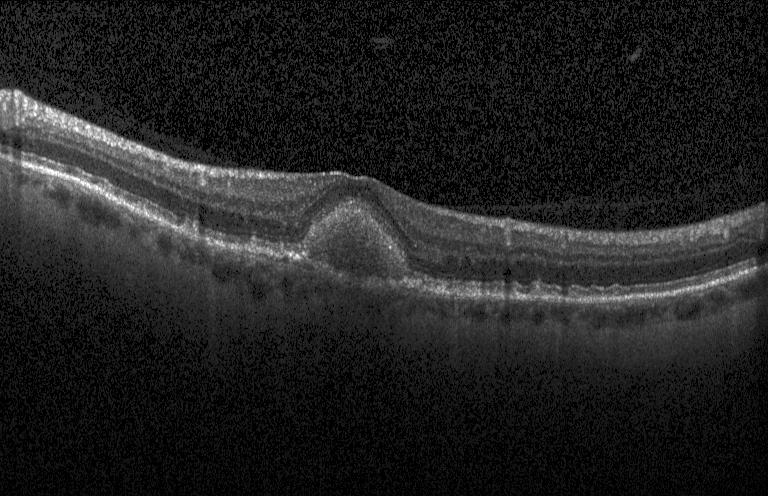

Diagnosis: choroidal neovascularization.